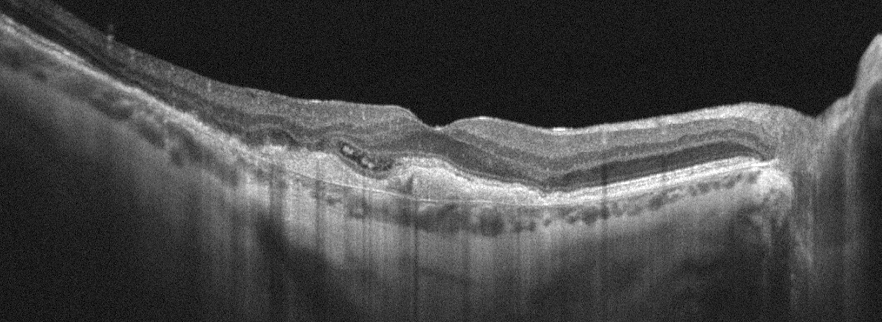
Acquired on an Optovue Avanti RTVue XR. Retinal OCT cross-section. Fovea-centered — Diagnosis: age-related macular degeneration (AMD).